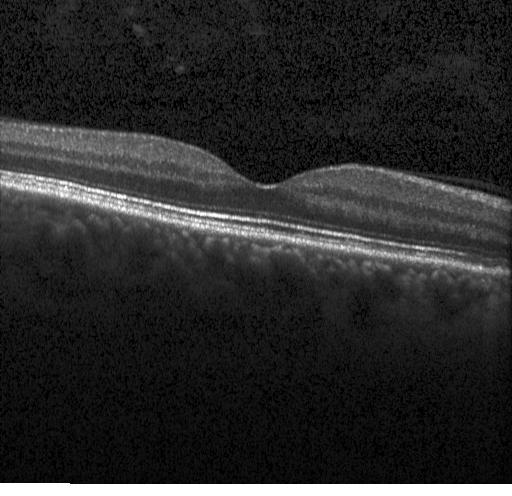
Impression: no choroidal neovascularization, no diabetic macular edema, and no drusen.